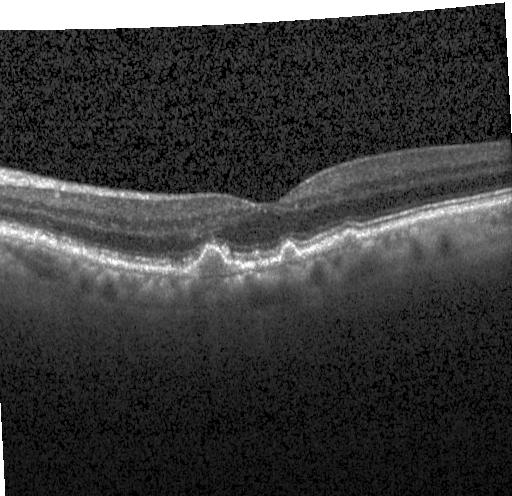
Impression: drusen.